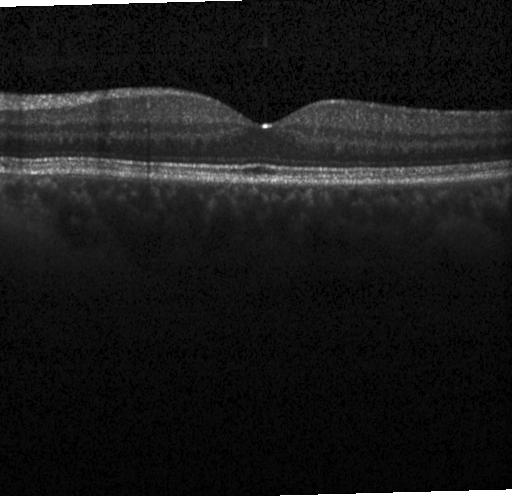

Optical coherence tomography B-scan. Macular scan. Instrument: Heidelberg Spectralis. Spectral-domain optical coherence tomography.
Neither choroidal neovascularization, diabetic macular edema, nor drusen.